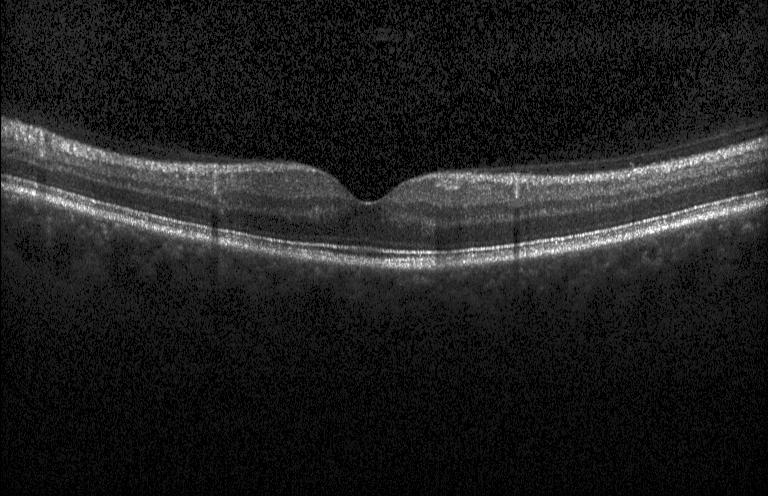 OCT B-scan; spectral-domain OCT; instrument: Heidelberg Spectralis.
Diagnosis: neither choroidal neovascularization, diabetic macular edema, nor drusen.